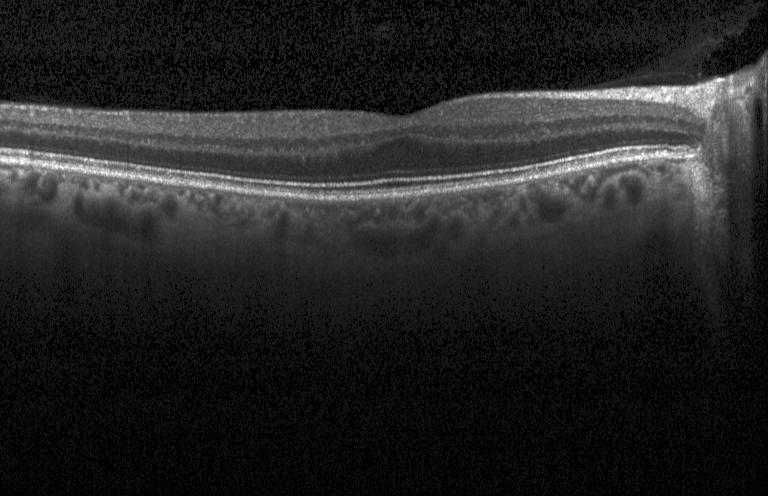 Finding: no choroidal neovascularization, no diabetic macular edema, and no drusen.